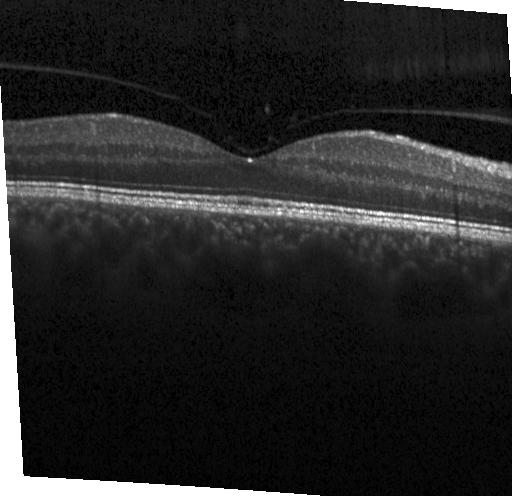 Heidelberg Spectralis OCT system. OCT line scan. Spectral-domain optical coherence tomography. Centered on the fovea.
Assessment: neither CNV, DME, nor drusen.